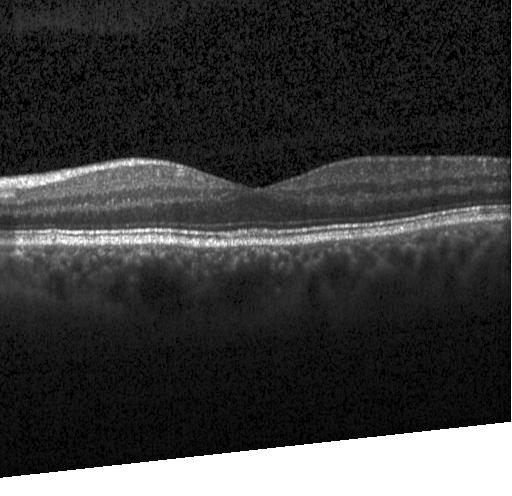 OCT finding: no CNV, DME, or drusen.